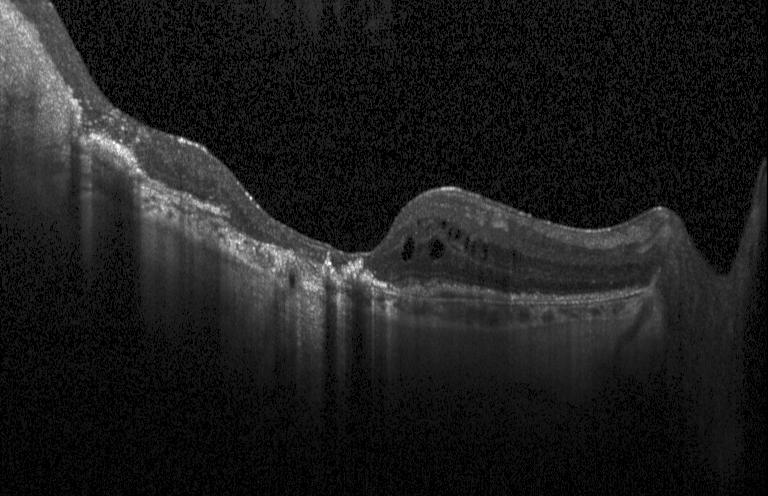 OCT line scan · spectral-domain optical coherence tomography
Macular OCT: a choroidal neovascular membrane.